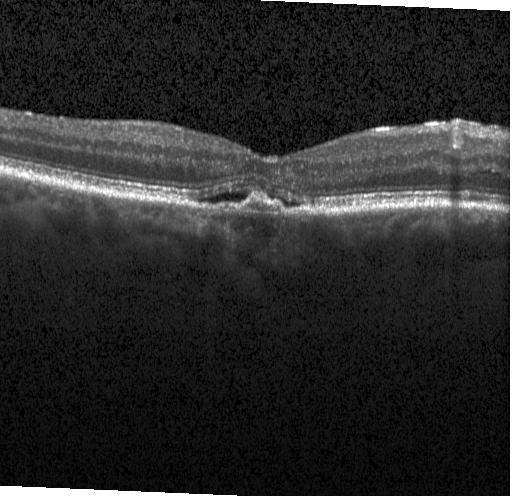
Retinal OCT cross-section · acquired on a Heidelberg Spectralis. Dx: choroidal neovascularization.